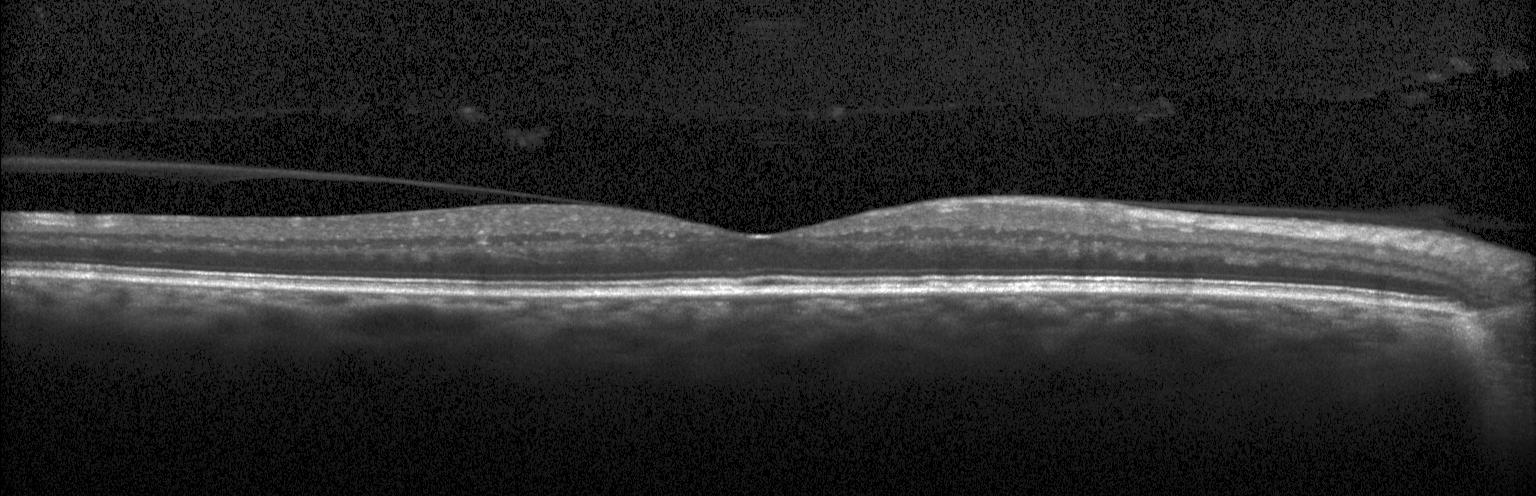 Heidelberg Spectralis OCT system; retinal OCT B-scan; horizontal scan through the fovea; SD-OCT. The scan shows no CNV, DME, or drusen.